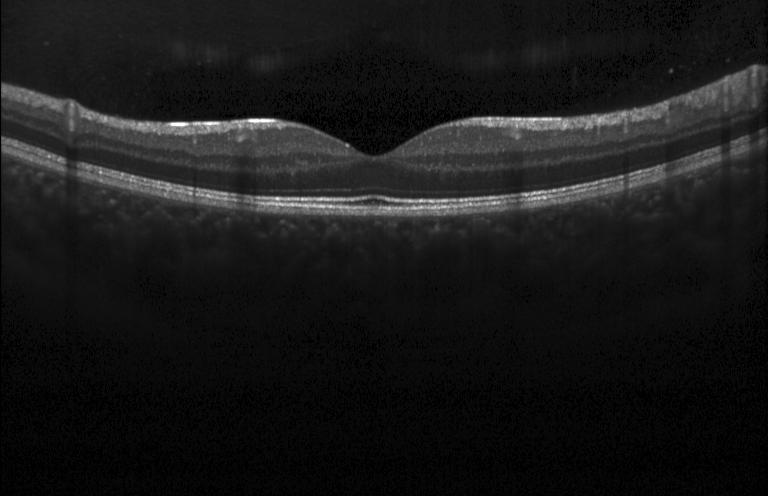 This B-scan demonstrates neither CNV, DME, nor drusen.